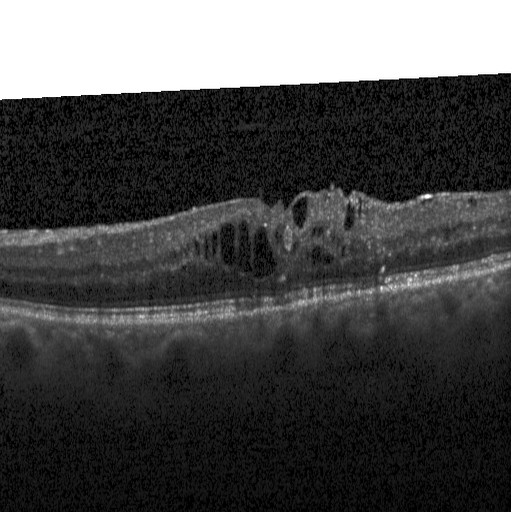 Impression: DME.